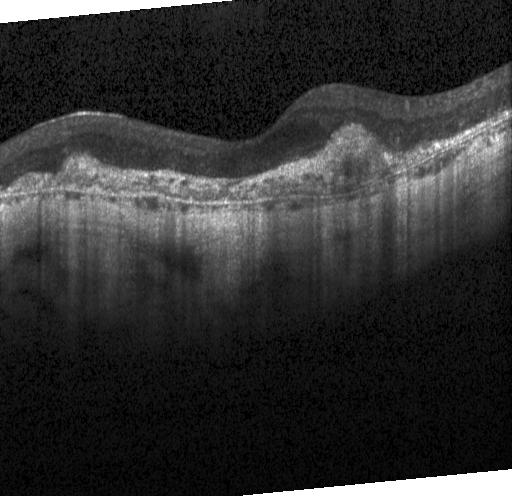
Instrument: Heidelberg Spectralis. Spectral-domain OCT. Fovea-centered. Retinal OCT B-scan.
This B-scan demonstrates a choroidal neovascular membrane.